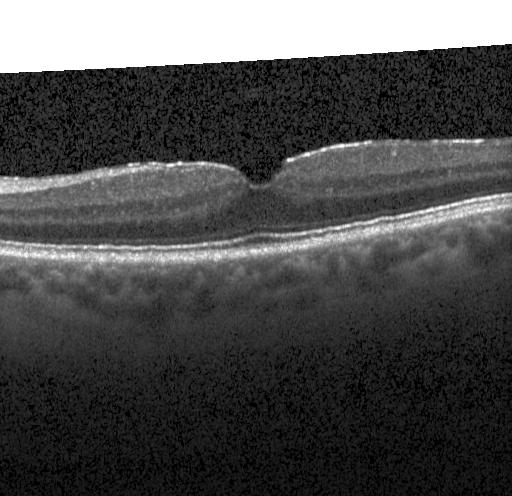

OCT scan showing no choroidal neovascularization, diabetic macular edema, or drusen.